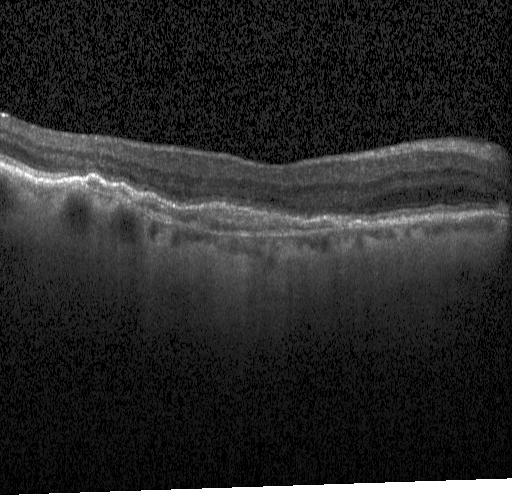 Instrument: Heidelberg Spectralis. Retinal OCT cross-section. Assessment: choroidal neovascularization (CNV).